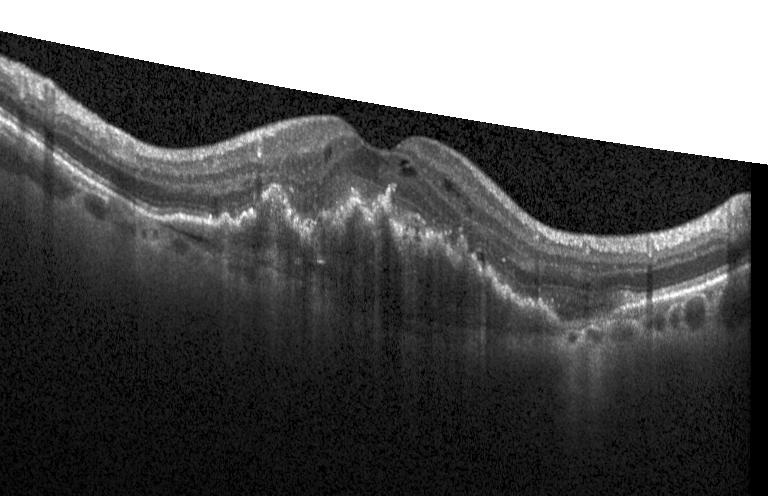

Impression: a choroidal neovascular membrane.